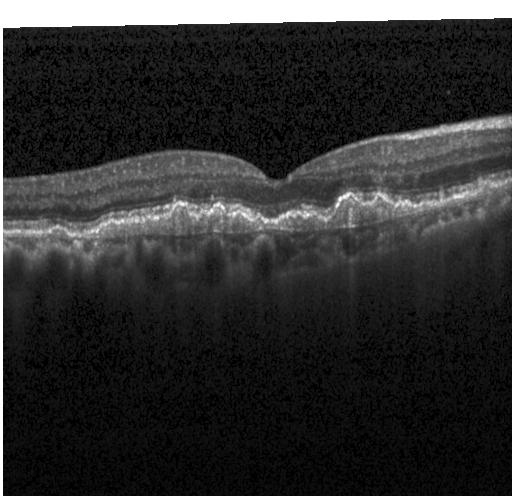 OCT finding: a choroidal neovascular membrane.